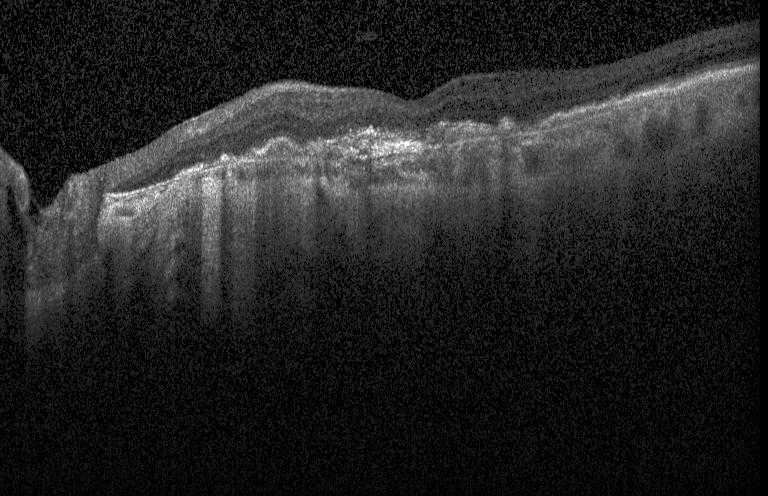 SD-OCT · retinal OCT B-scan.
Finding: choroidal neovascularization (CNV).